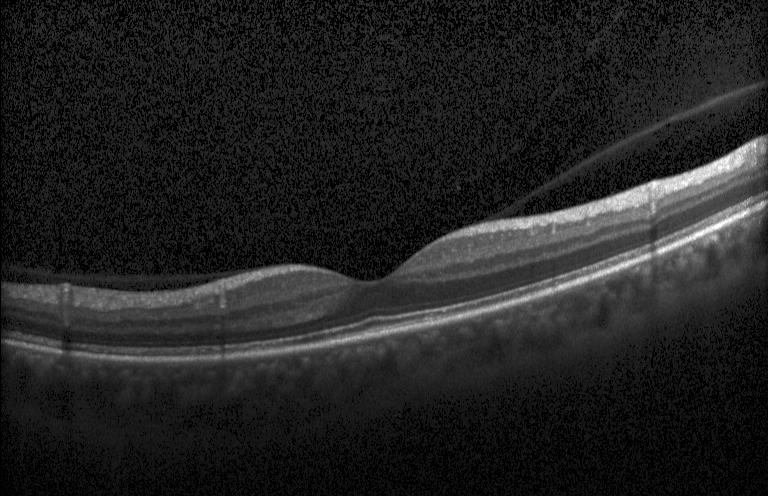 Dx: no CNV, DME, or drusen.